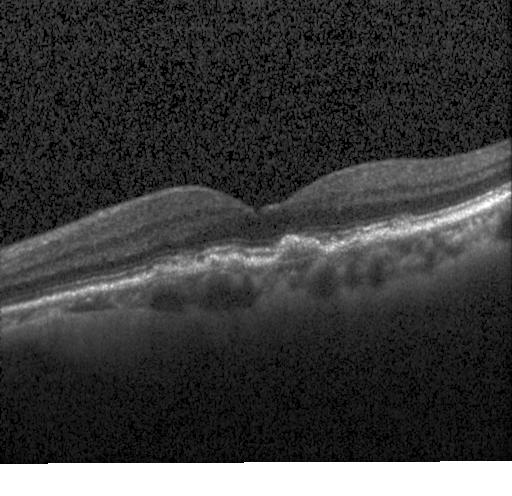
Acquired on a Heidelberg Spectralis; OCT B-scan — Diagnosis: sub-RPE drusenoid deposits.